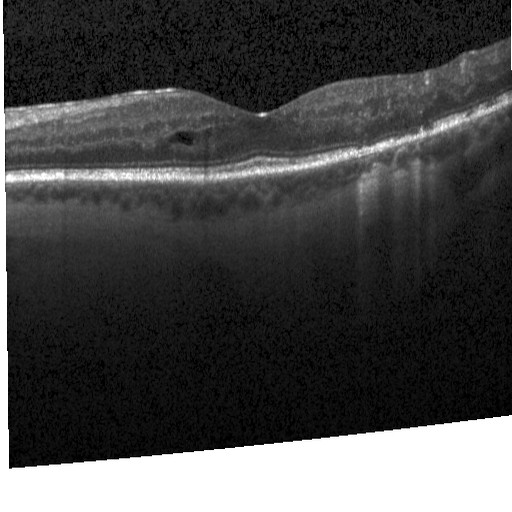

Optical coherence tomography scan. Impression: diabetic macular edema.